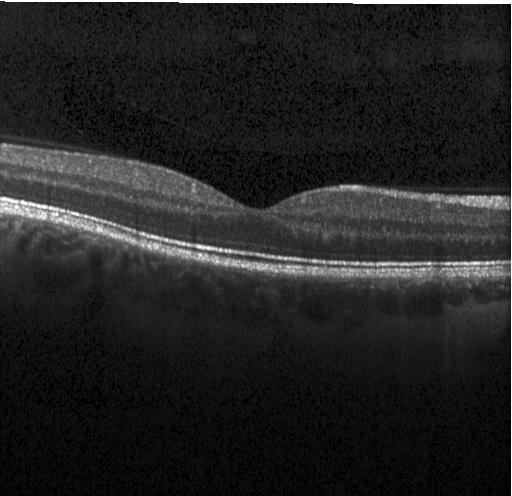

Optical coherence tomography B-scan.
OCT finding: no choroidal neovascularization, no diabetic macular edema, and no drusen.